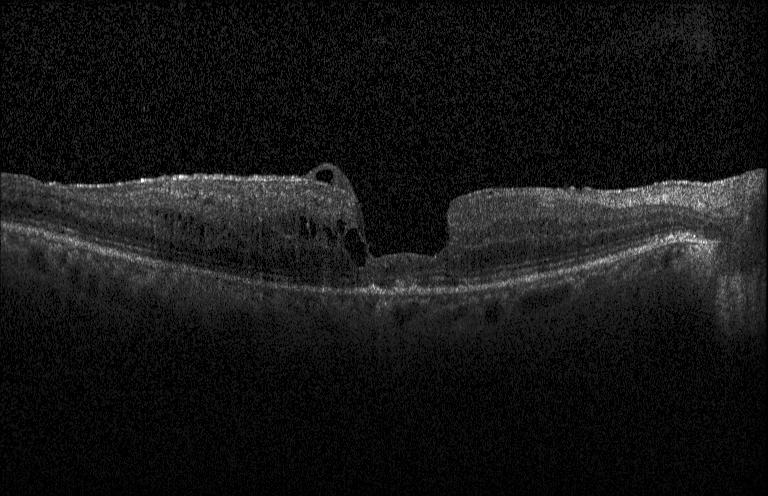 Acquired on a Heidelberg Spectralis; retinal OCT B-scan; spectral-domain OCT
OCT finding: diabetic macular edema.